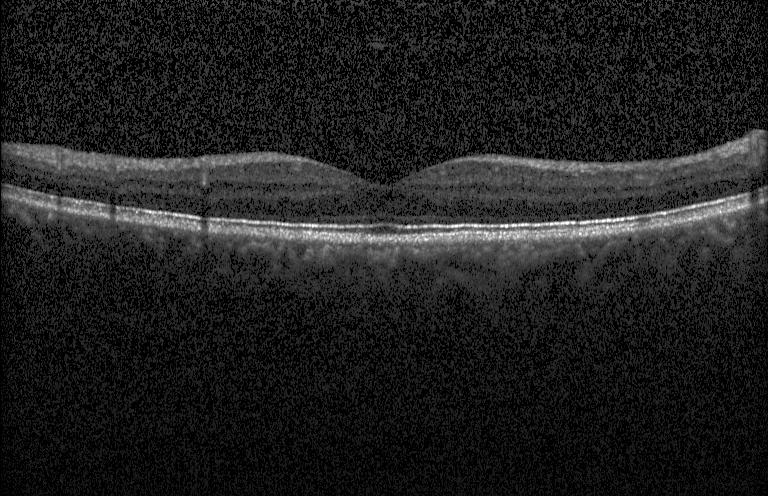 Optical coherence tomography scan — The scan shows no CNV, DME, or drusen.